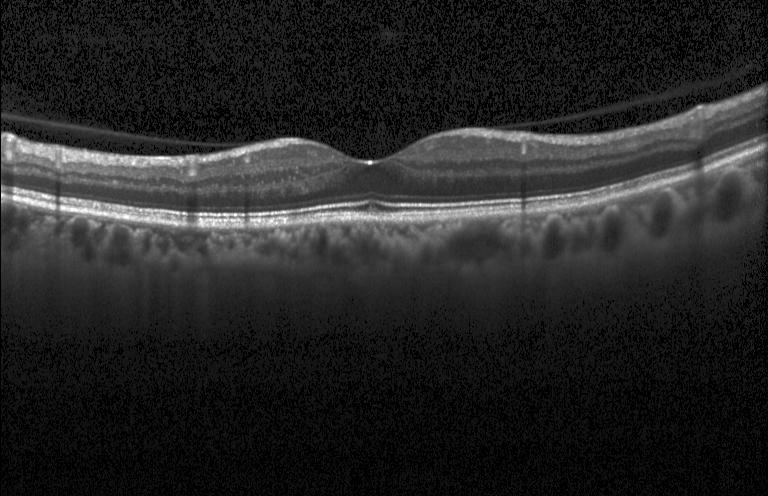
Finding: neither choroidal neovascularization, diabetic macular edema, nor drusen.